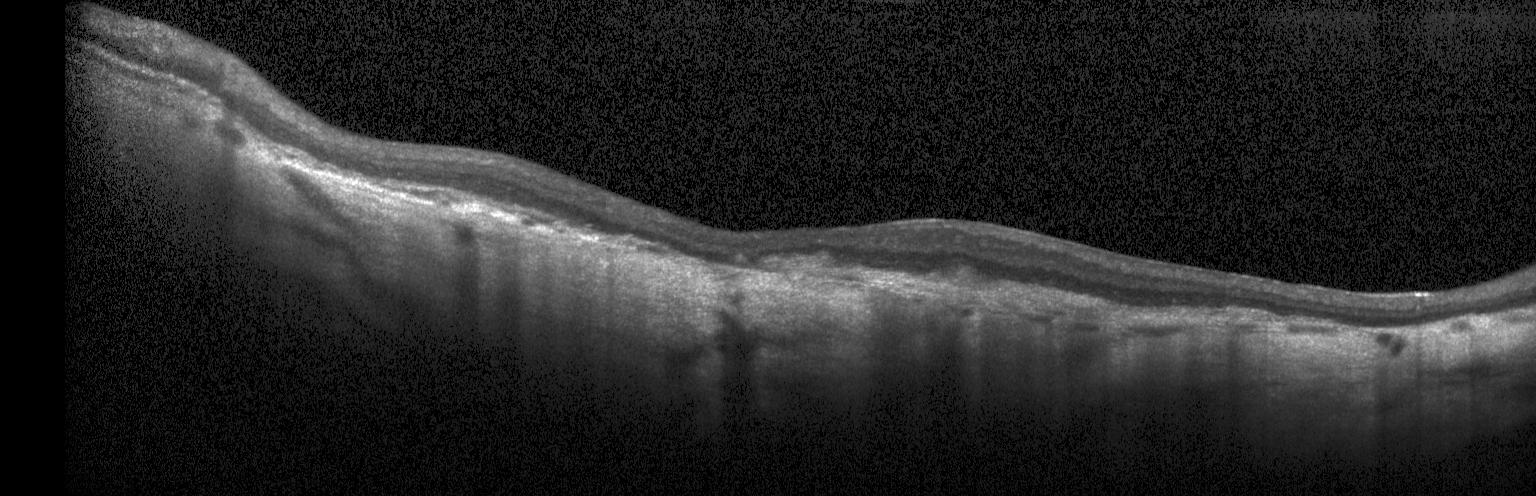
A choroidal neovascular membrane.